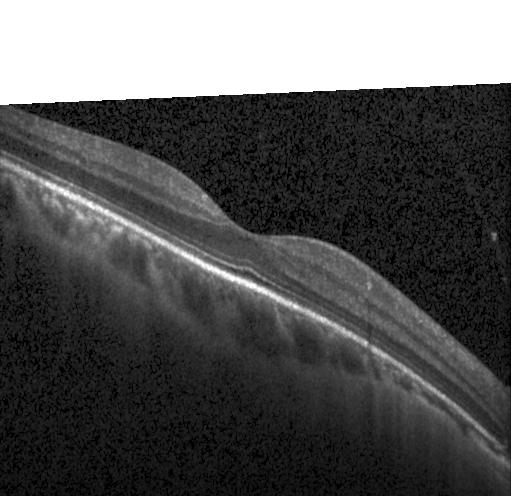 Fovea-centered, optical coherence tomography B-scan, Heidelberg Spectralis, spectral-domain OCT. The scan shows no evidence of choroidal neovascularization, diabetic macular edema, or drusen.